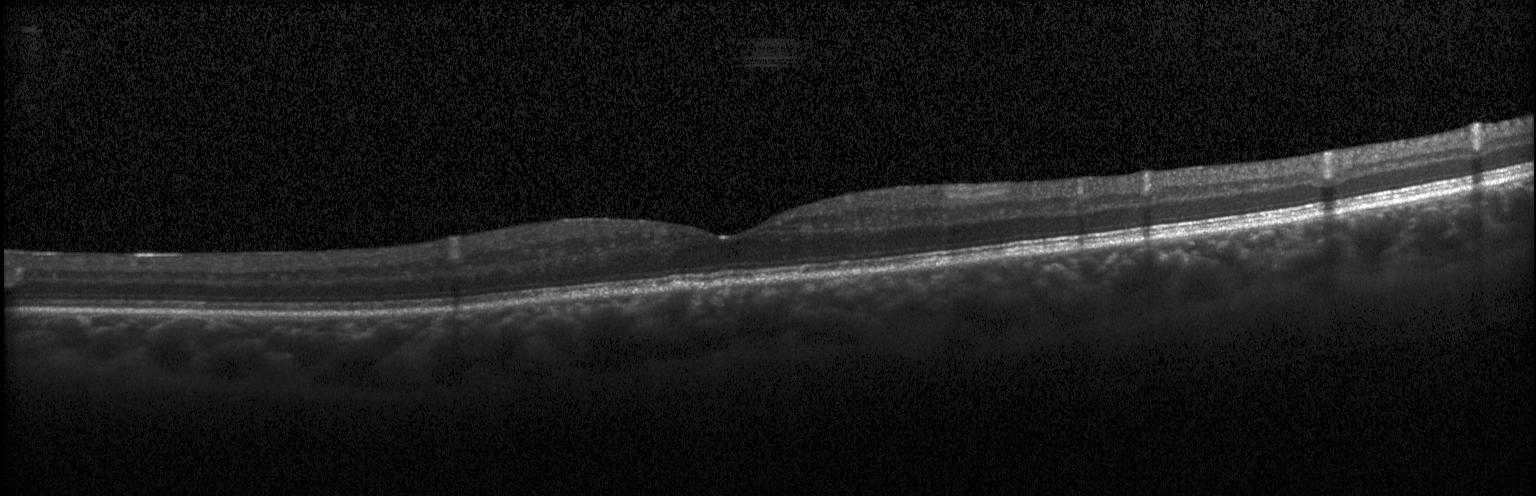

The scan shows no evidence of CNV, DME, or drusen.